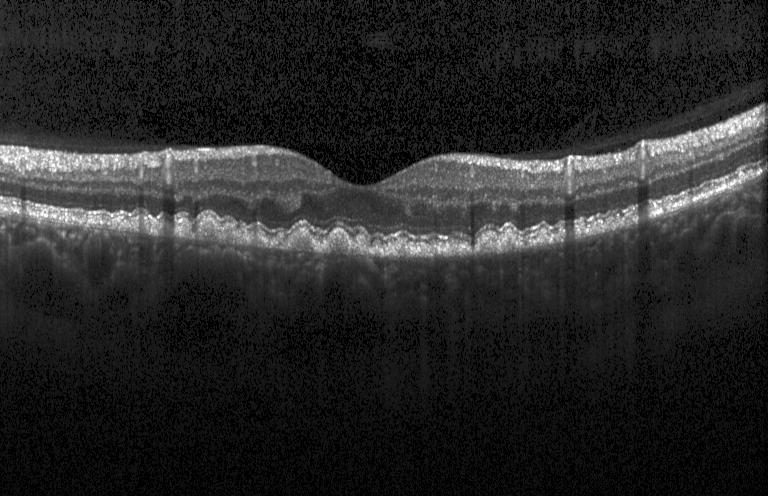
OCT line scan
Impression: multiple drusen.